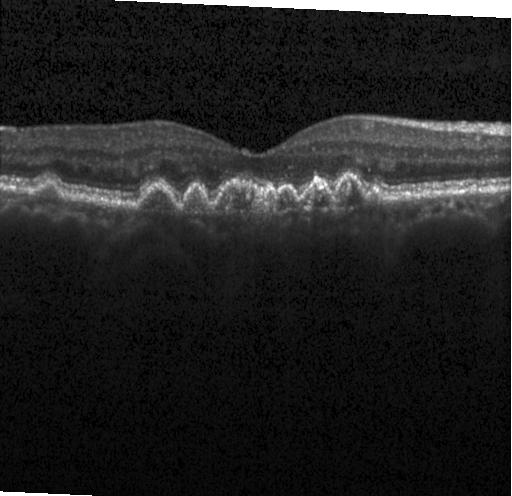 Centered on the fovea, spectral-domain OCT, optical coherence tomography scan.
A choroidal neovascular membrane.